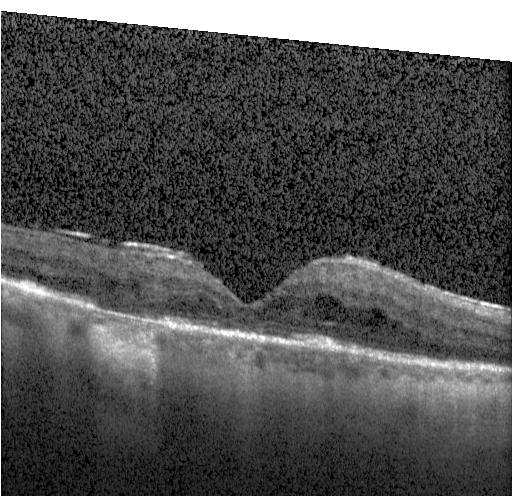 Horizontal scan through the fovea. OCT B-scan. Heidelberg Spectralis OCT system. Spectral-domain optical coherence tomography
Diabetic macular edema.